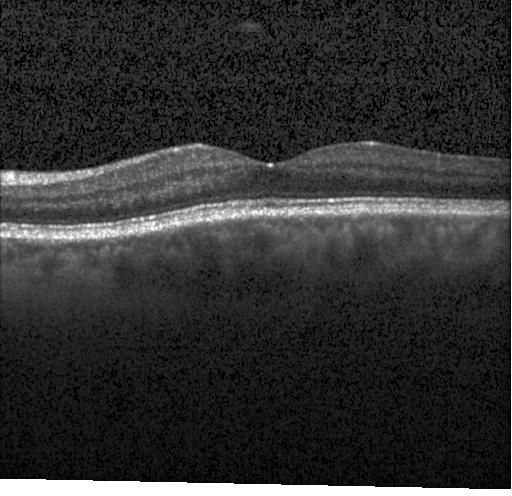

Spectral-domain optical coherence tomography; fovea-centered; retinal OCT B-scan; acquired on a Heidelberg Spectralis. Macular OCT: no CNV, DME, or drusen.